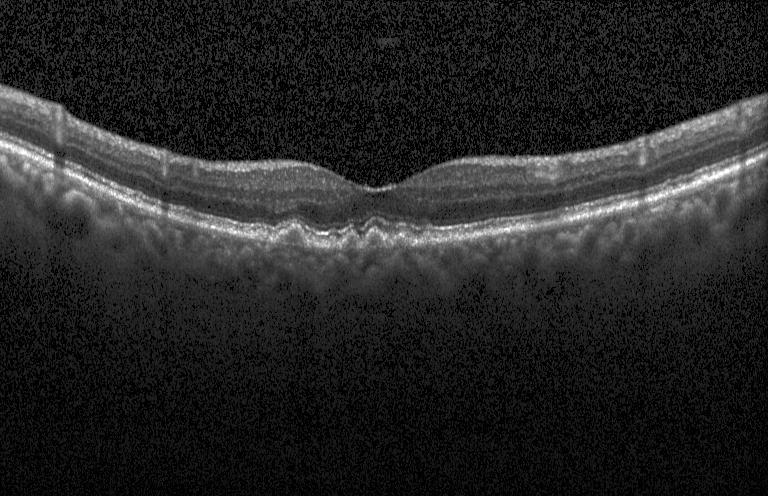
OCT finding: drusen.